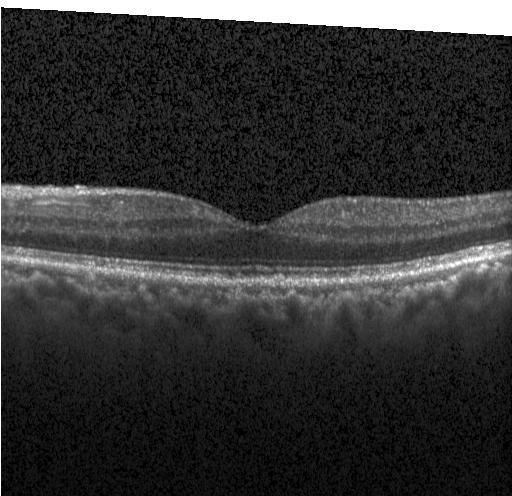

Retinal OCT B-scan; macular scan; SD-OCT. Diagnosis: no evidence of choroidal neovascularization, diabetic macular edema, or drusen.